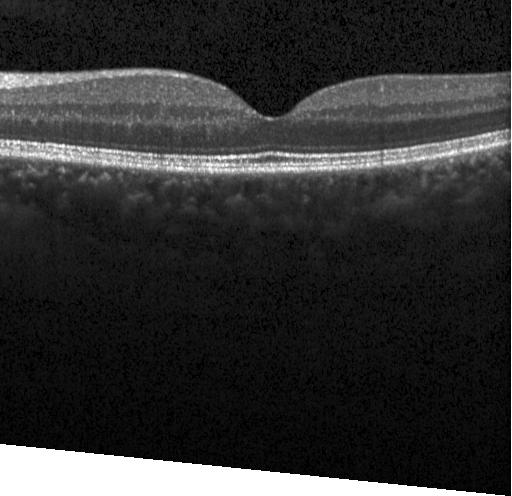

Acquired on a Heidelberg Spectralis; optical coherence tomography B-scan
Impression: neither choroidal neovascularization, diabetic macular edema, nor drusen.